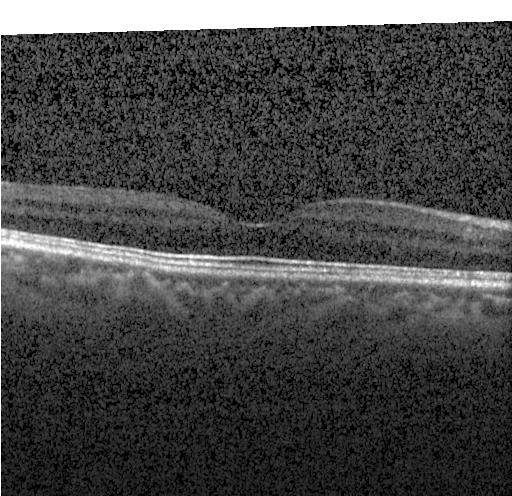

Optical coherence tomography scan — OCT finding: no evidence of choroidal neovascularization, diabetic macular edema, or drusen.